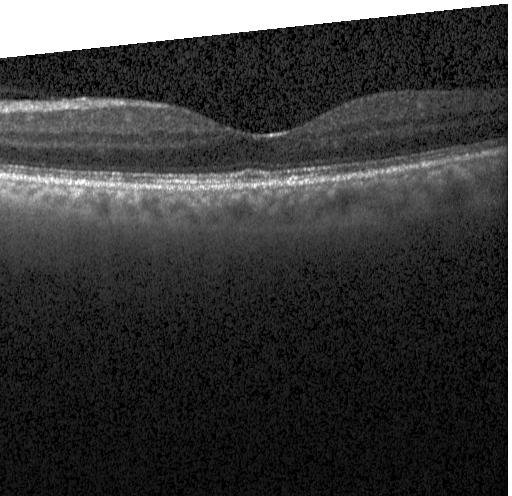 Optical coherence tomography B-scan.
OCT finding: no evidence of CNV, DME, or drusen.